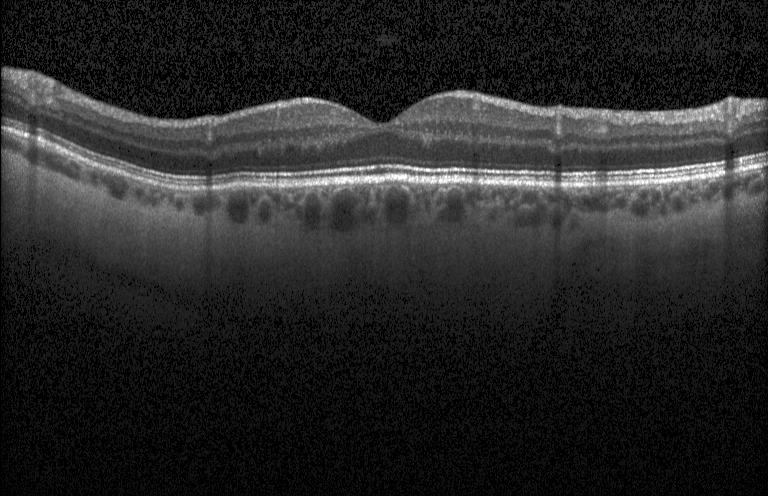
Heidelberg Spectralis OCT system; retinal OCT cross-section; centered on the fovea; spectral-domain optical coherence tomography — Macular OCT: no choroidal neovascularization, diabetic macular edema, or drusen.